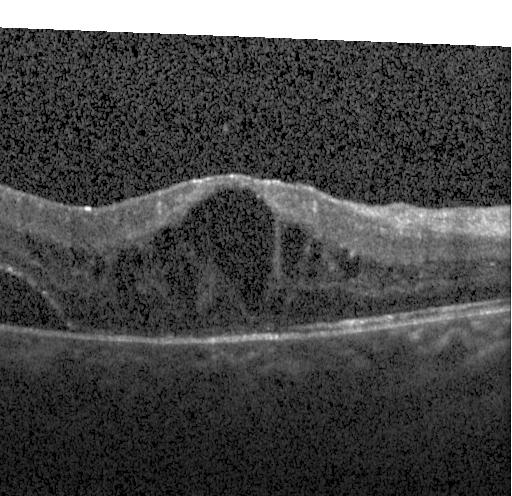

Macular scan. Optical coherence tomography scan.
Assessment: DME.